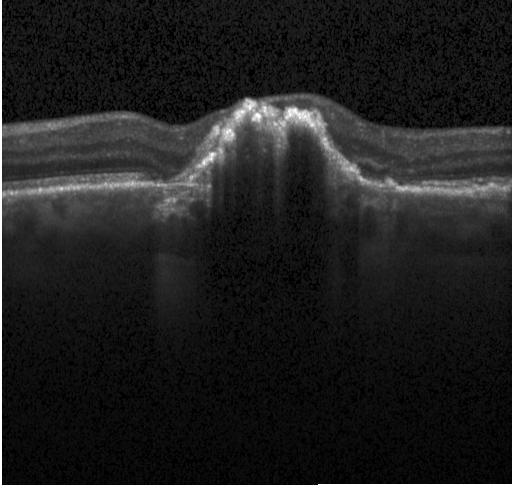

Optical coherence tomography B-scan. Acquired on a Heidelberg Spectralis. Through the macula.
Impression: a choroidal neovascular membrane.